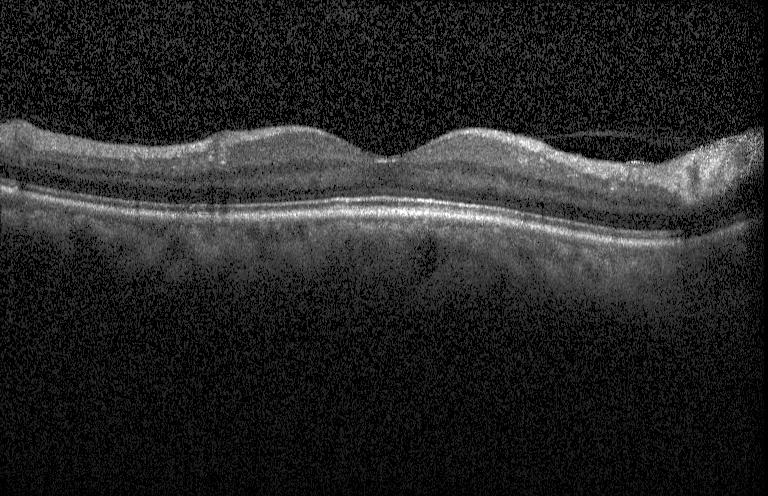 Heidelberg Spectralis OCT system; optical coherence tomography scan; SD-OCT; horizontal scan through the fovea.
Finding: no evidence of CNV, DME, or drusen.